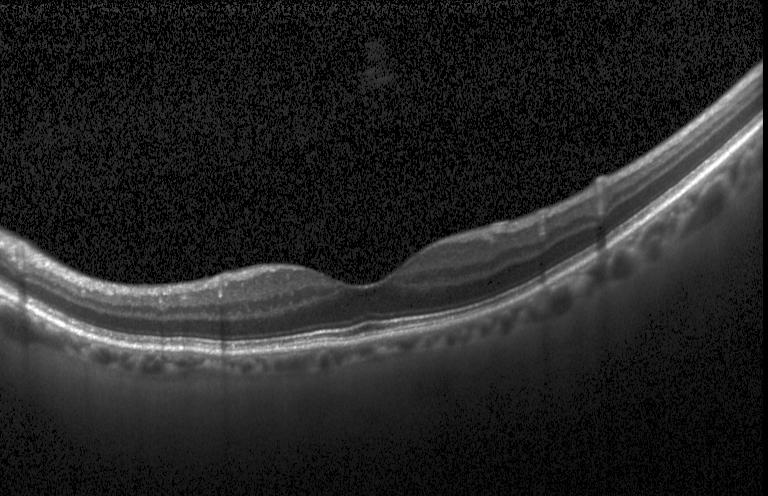

Optical coherence tomography scan · fovea-centered — Dx: neither choroidal neovascularization, diabetic macular edema, nor drusen.